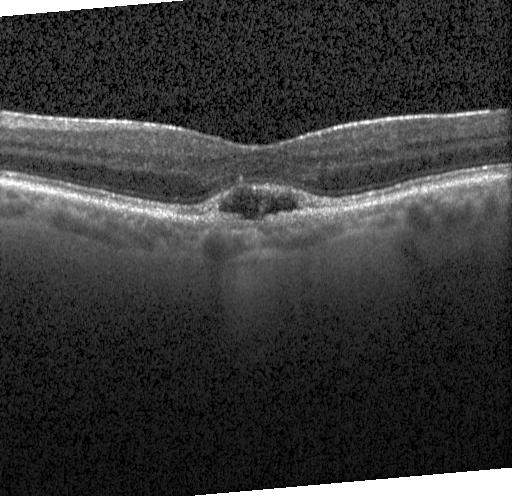
Optical coherence tomography B-scan · spectral-domain optical coherence tomography · fovea-centered. Dx: a choroidal neovascular membrane.